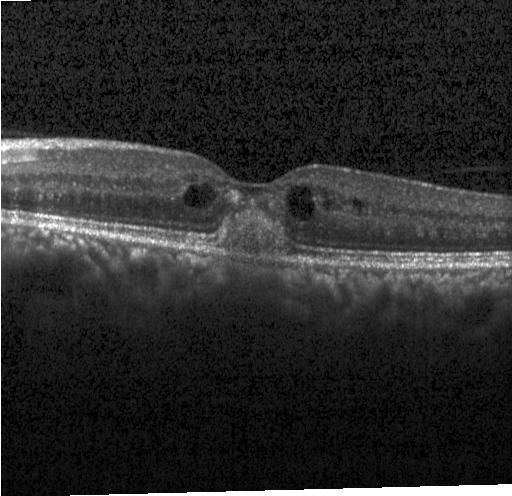
OCT B-scan
Diagnosis: a choroidal neovascular membrane.